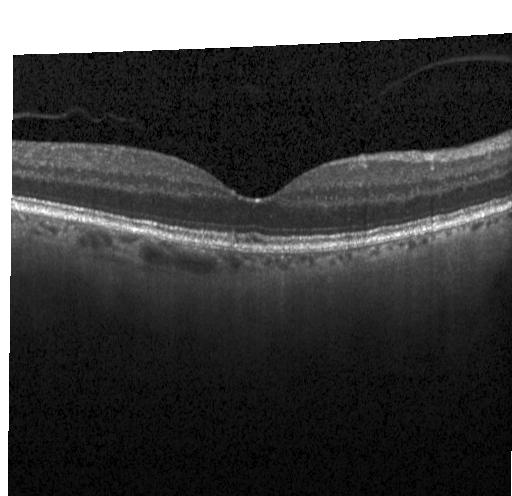 Optical coherence tomography B-scan
Macular OCT: no CNV, no DME, and no drusen.